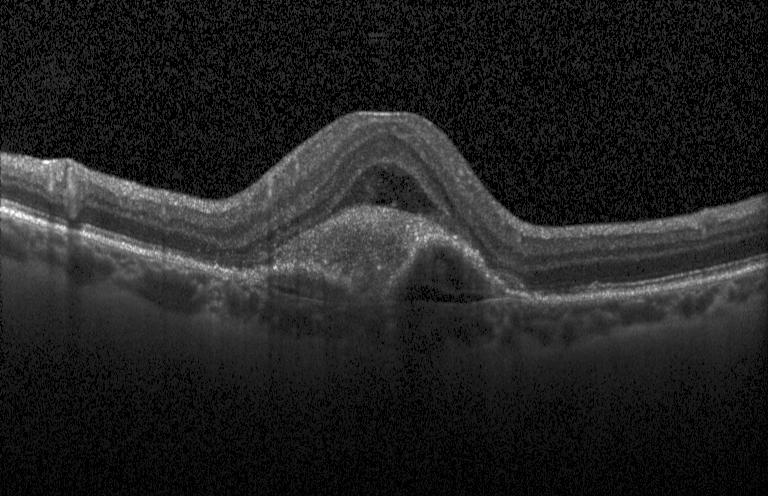
Through the macula, retinal OCT B-scan. Impression: a choroidal neovascular membrane.